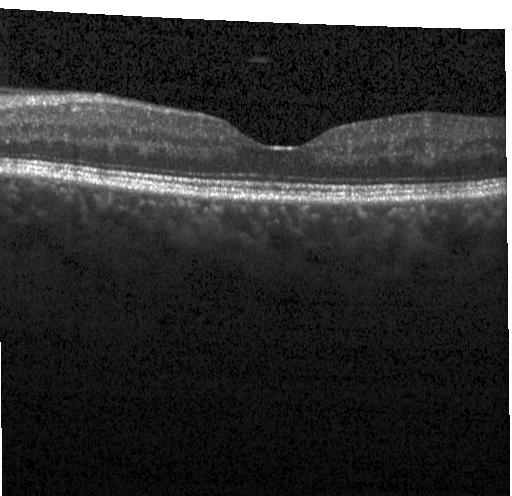
Retinal OCT B-scan — Assessment: no choroidal neovascularization, diabetic macular edema, or drusen.